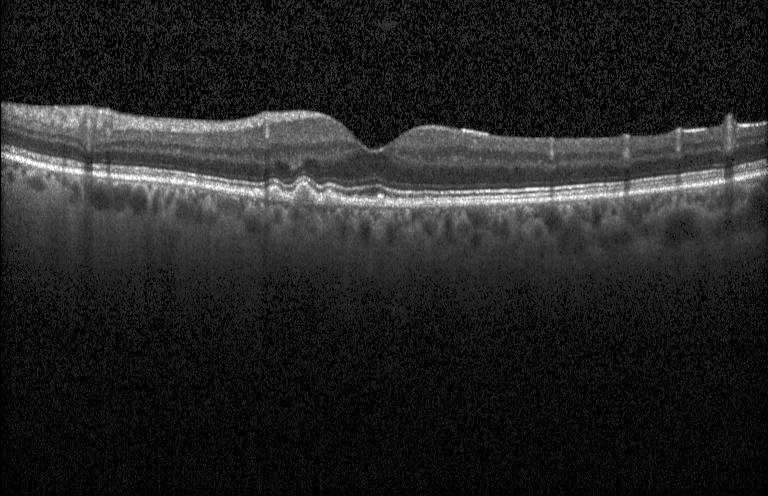

OCT finding: drusen.